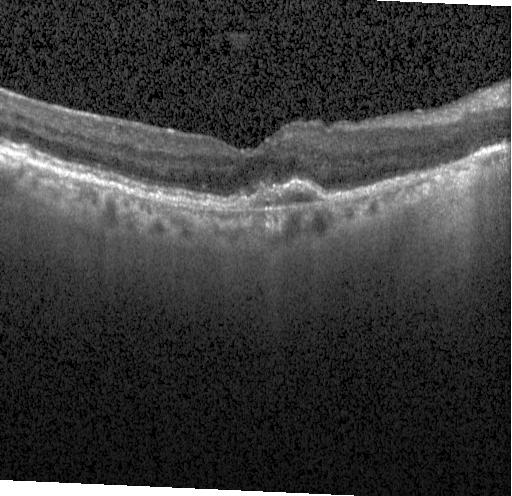 OCT B-scan showing CNV.